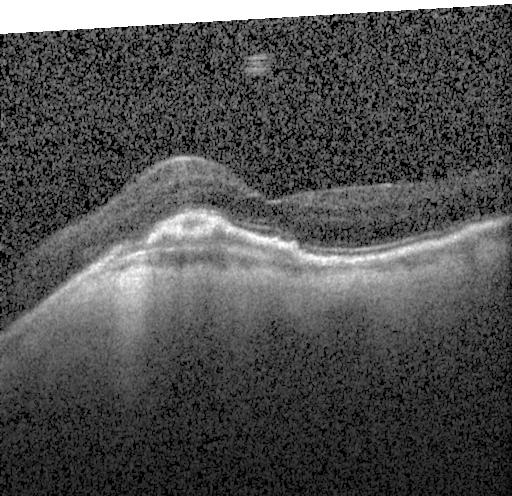
Impression: a choroidal neovascular membrane.